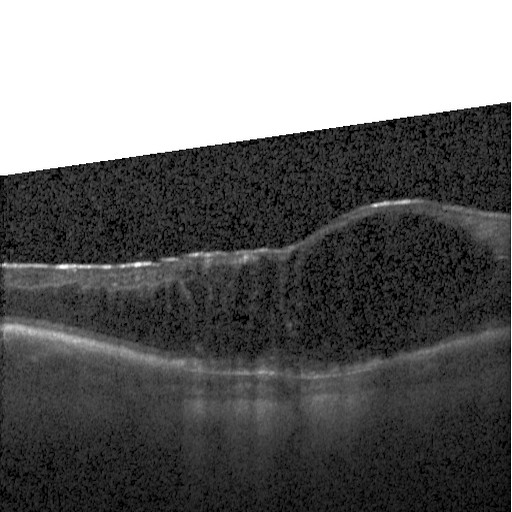 Impression: diabetic macular edema.